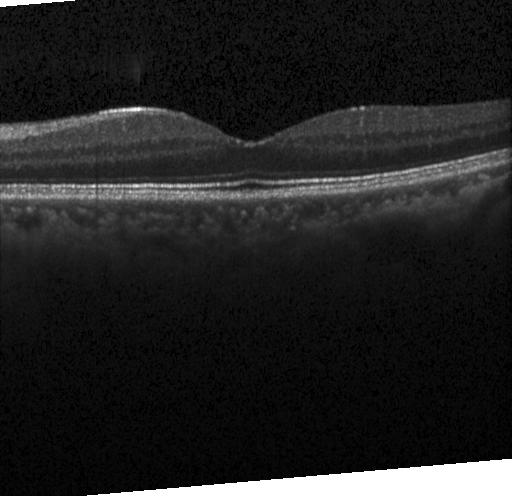

Retinal OCT B-scan, through the macula.
Diagnosis: neither choroidal neovascularization, diabetic macular edema, nor drusen.